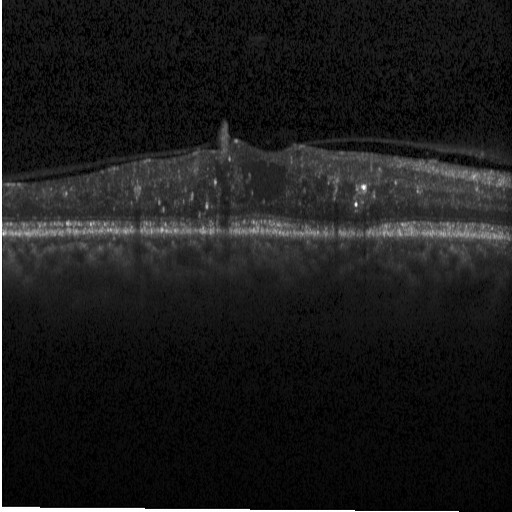
OCT B-scan, spectral-domain OCT, acquired on a Heidelberg Spectralis.
Assessment: DME.